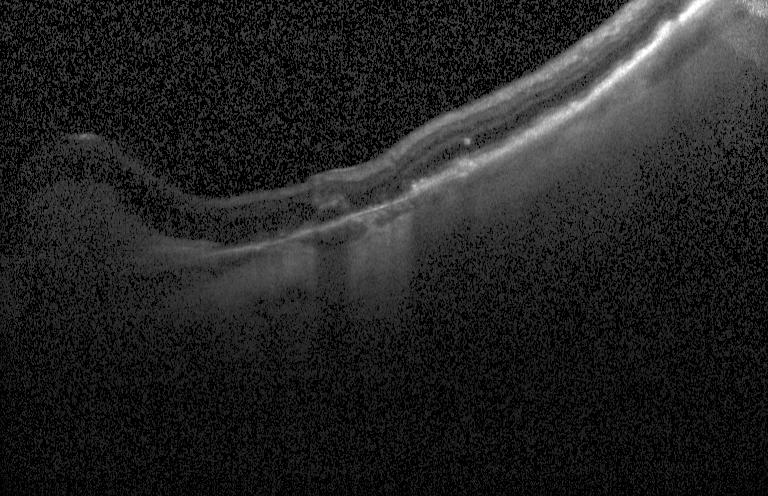

Spectral-domain OCT, Heidelberg Spectralis OCT system, optical coherence tomography B-scan. This B-scan demonstrates a choroidal neovascular membrane.